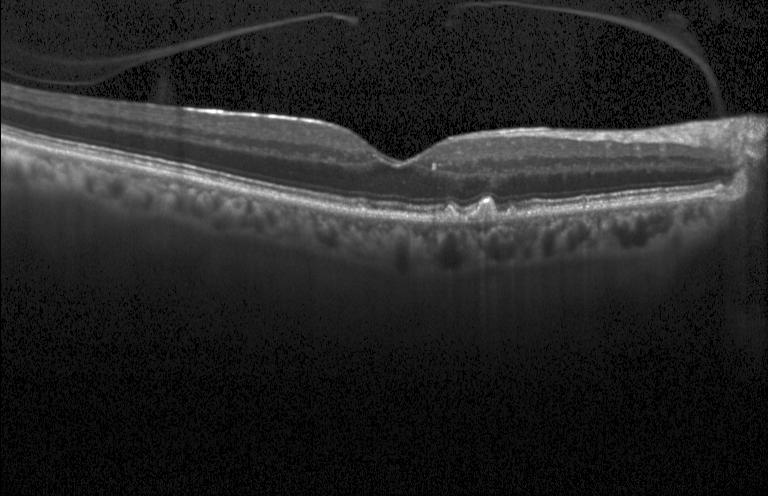
Diagnosis: multiple drusen.